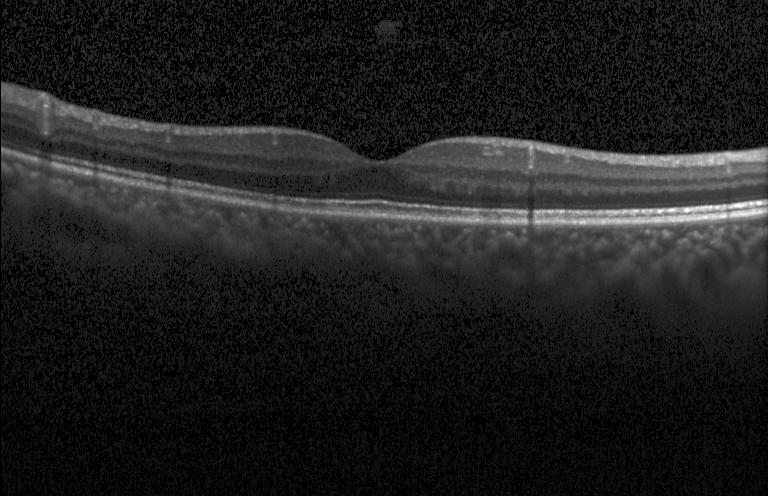 Macular scan, OCT line scan — OCT finding: no evidence of choroidal neovascularization, diabetic macular edema, or drusen.